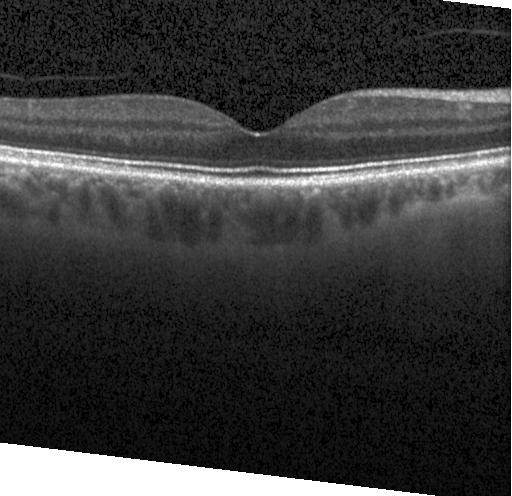
Macular OCT: no evidence of CNV, DME, or drusen.